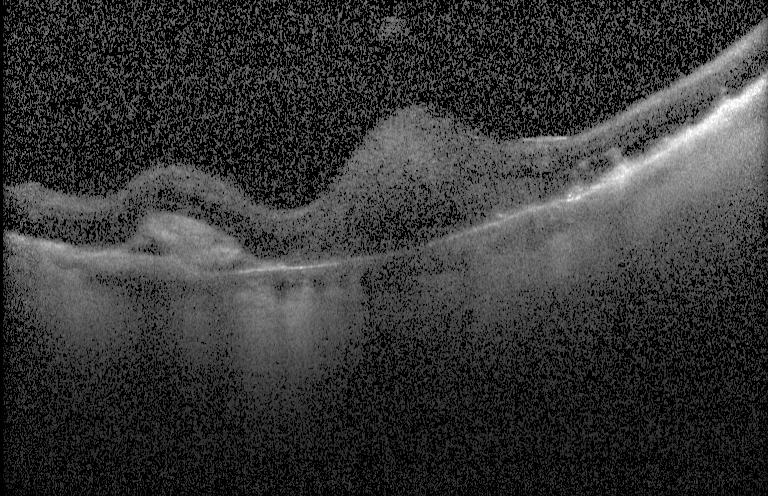
Retinal OCT cross-section; spectral-domain optical coherence tomography. Finding: a choroidal neovascular membrane.